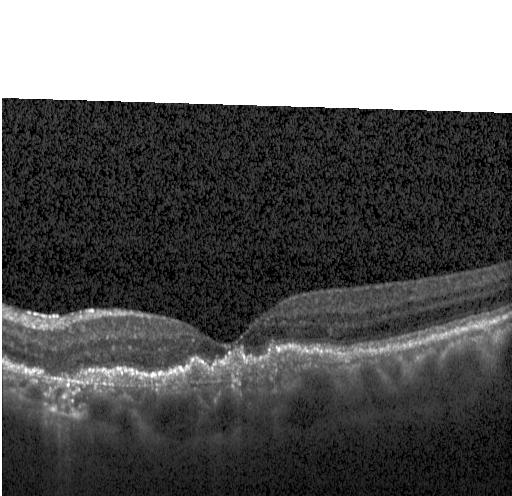 Dx: choroidal neovascularization (CNV).